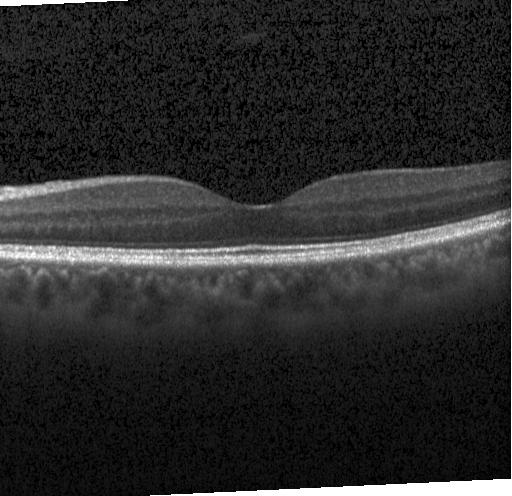

Acquired on a Heidelberg Spectralis; optical coherence tomography scan
Macular OCT: no evidence of choroidal neovascularization, diabetic macular edema, or drusen.